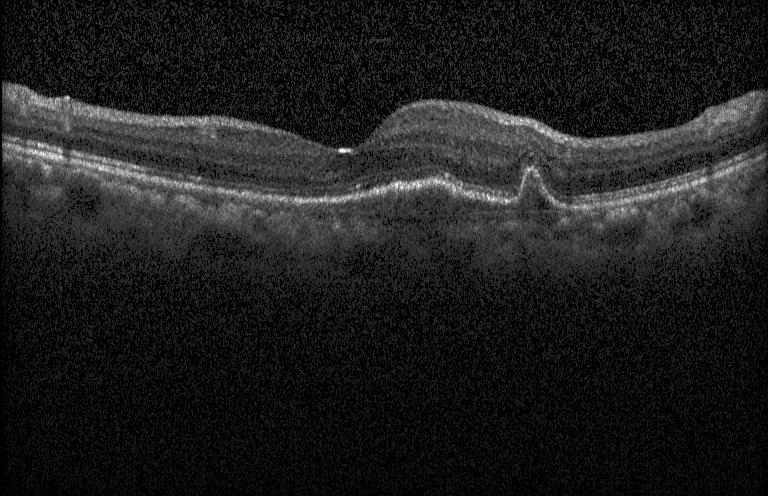
Optical coherence tomography B-scan
Macular OCT: a choroidal neovascular membrane.